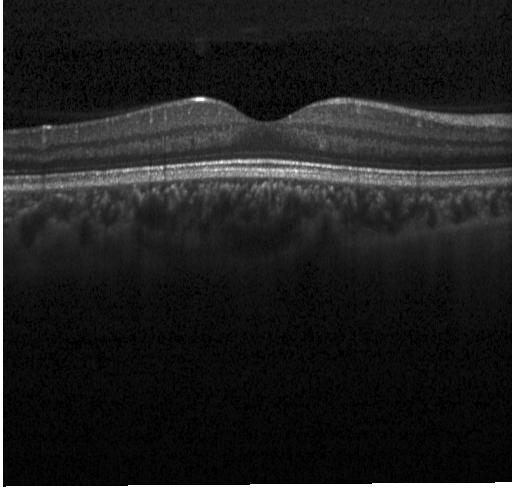
OCT line scan · spectral-domain optical coherence tomography
Dx: neither choroidal neovascularization, diabetic macular edema, nor drusen.